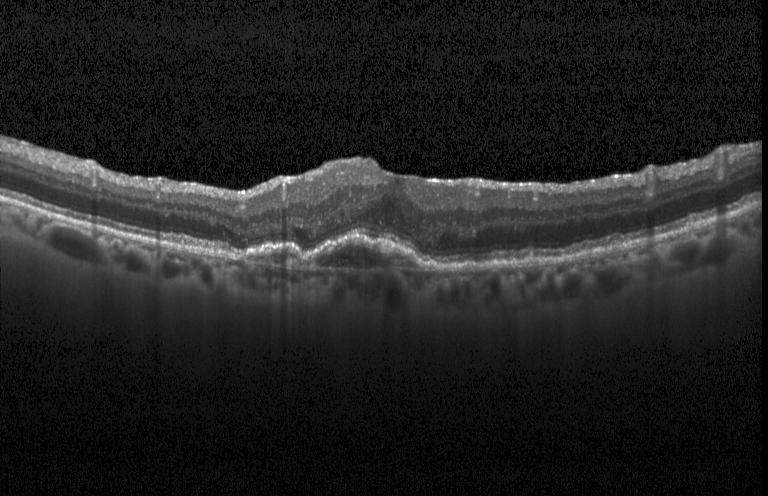
Finding: a choroidal neovascular membrane.